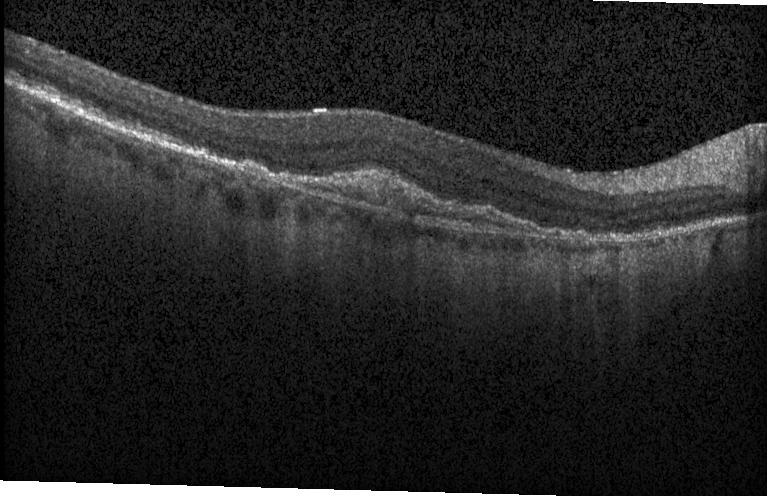

Instrument: Heidelberg Spectralis; spectral-domain OCT; retinal OCT B-scan. Macular OCT: a choroidal neovascular membrane.